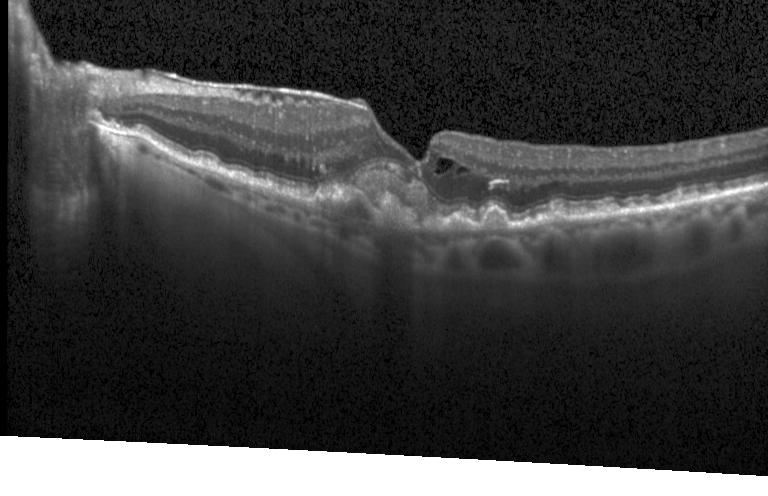
Through the macula, spectral-domain OCT, retinal OCT B-scan, Heidelberg Spectralis OCT system — Finding: choroidal neovascularization (CNV).